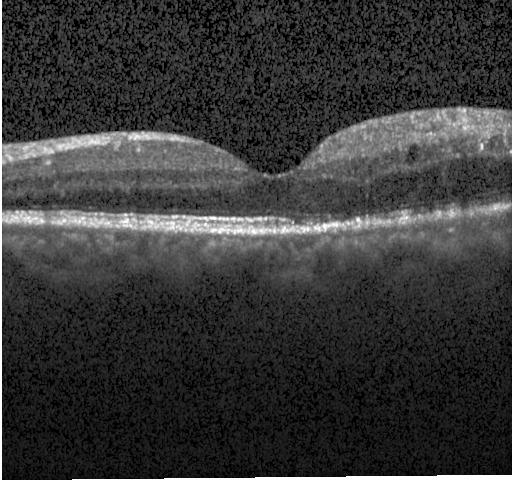 Assessment: DME.